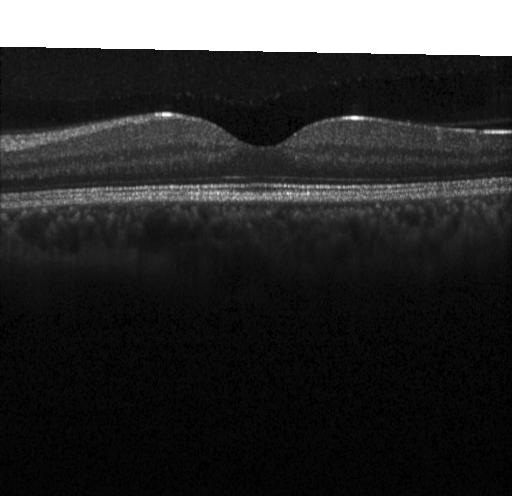

Macular OCT demonstrating no CNV, no DME, and no drusen.